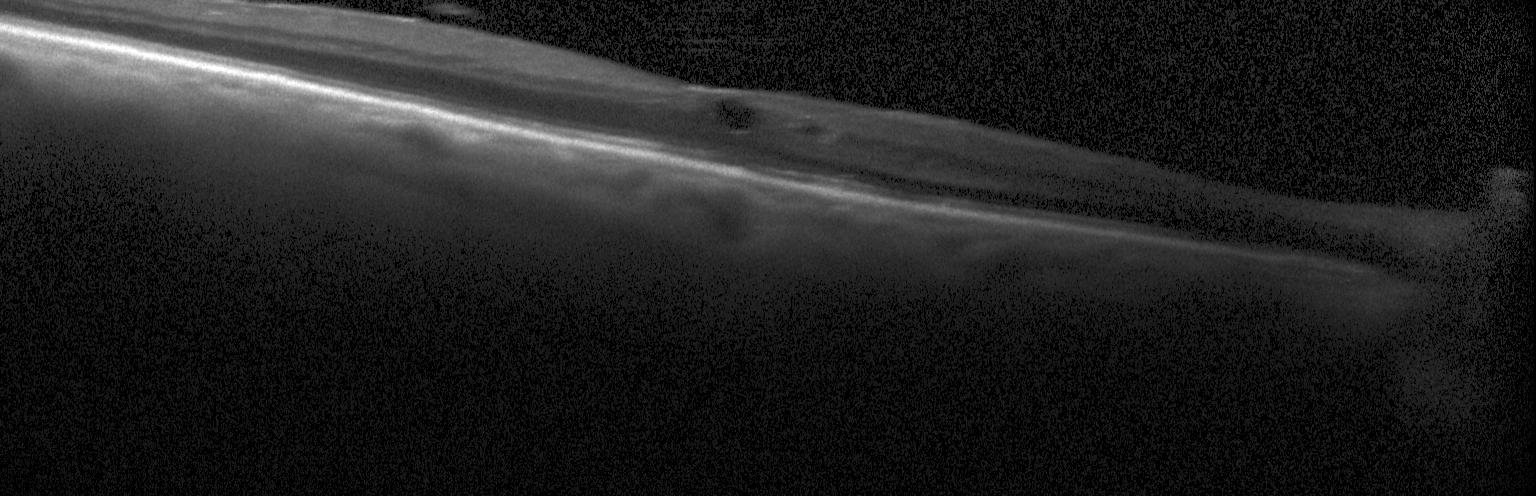

Spectral-domain optical coherence tomography, retinal OCT B-scan
Diagnosis: diabetic macular edema (DME).